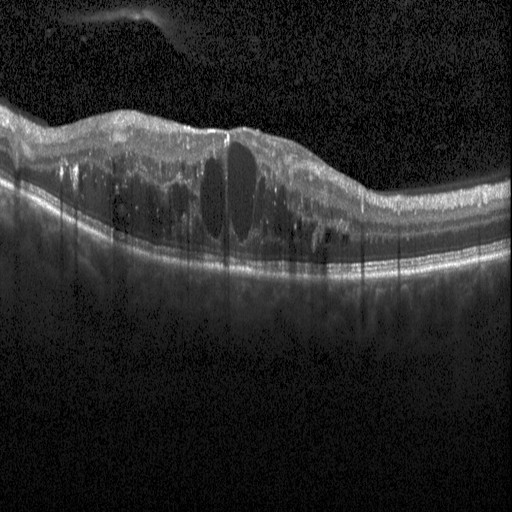

The scan shows DME.